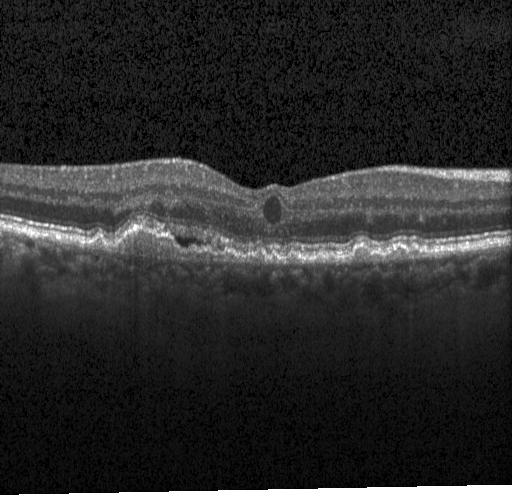 Instrument: Heidelberg Spectralis, fovea-centered, retinal OCT B-scan, spectral-domain OCT.
Assessment: a choroidal neovascular membrane.